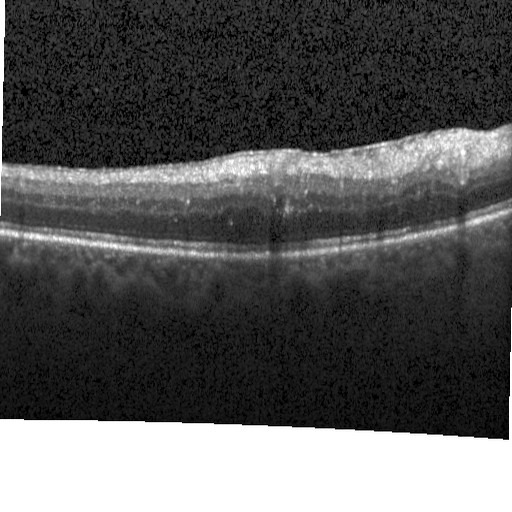 Dx: DME.